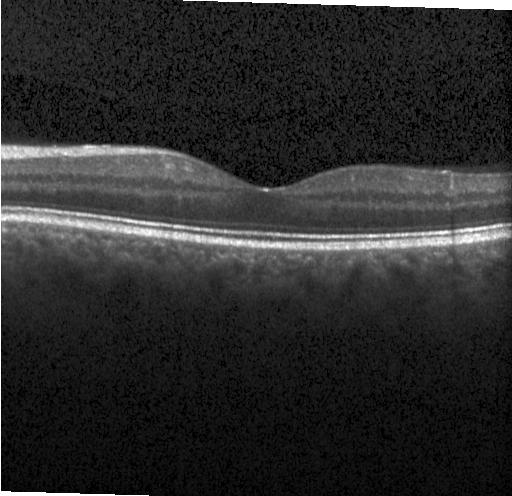
Spectral-domain OCT; horizontal scan through the fovea; Heidelberg Spectralis OCT system; retinal OCT cross-section. Assessment: no evidence of choroidal neovascularization, diabetic macular edema, or drusen.